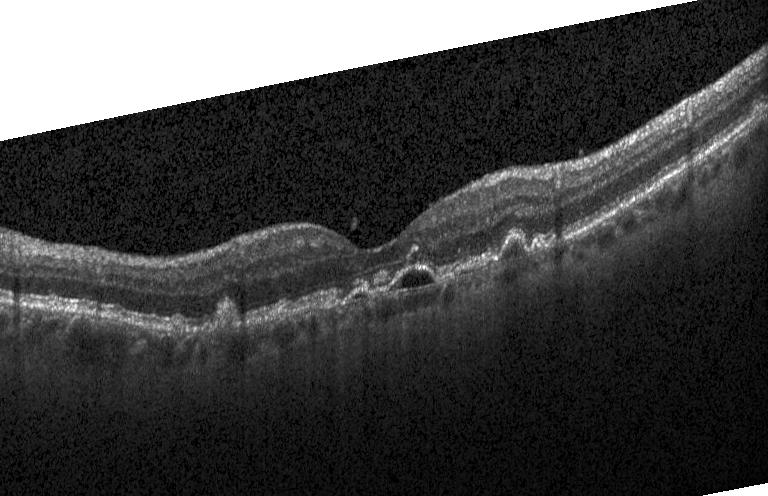

Dx: choroidal neovascularization (CNV).